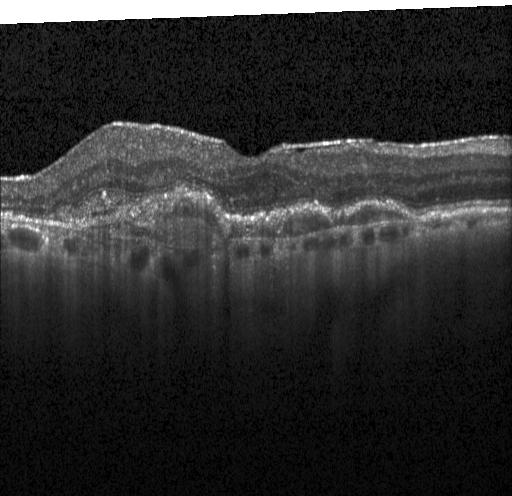
Spectral-domain optical coherence tomography. Acquired on a Heidelberg Spectralis. Horizontal scan through the fovea. OCT line scan.
Assessment: a choroidal neovascular membrane.